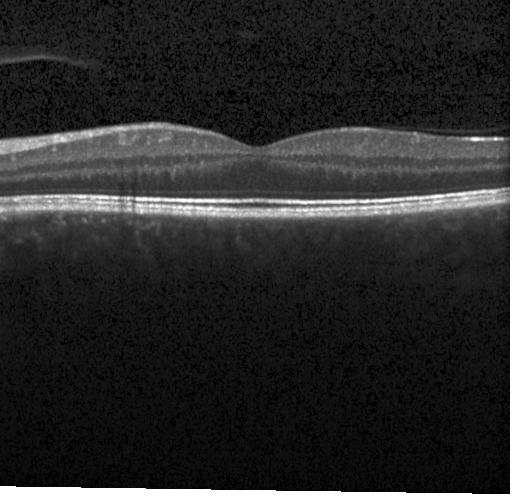

Impression: no CNV, no DME, and no drusen.